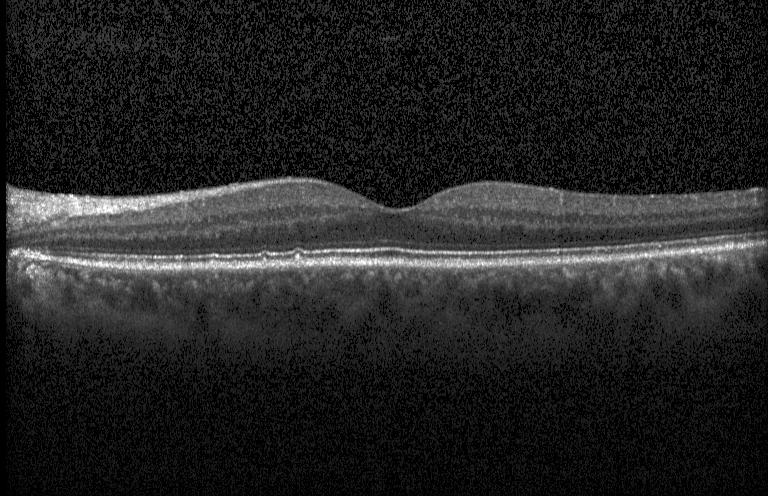

Retinal OCT B-scan.
Dx: drusen.